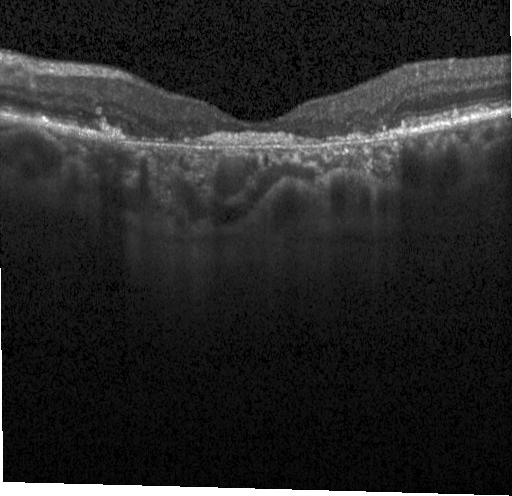

Impression: choroidal neovascularization (CNV).